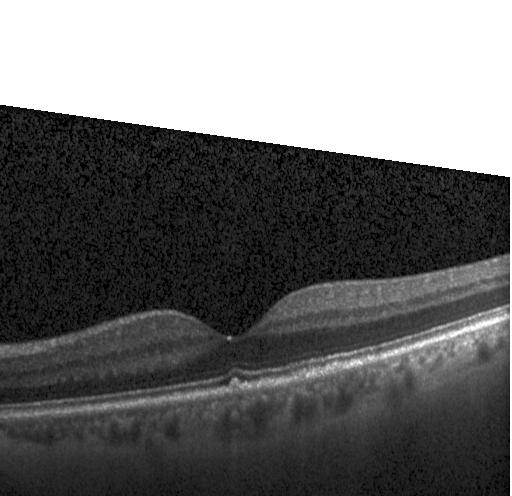
Centered on the fovea, retinal OCT cross-section, instrument: Heidelberg Spectralis, spectral-domain optical coherence tomography.
Diagnosis: multiple drusen.